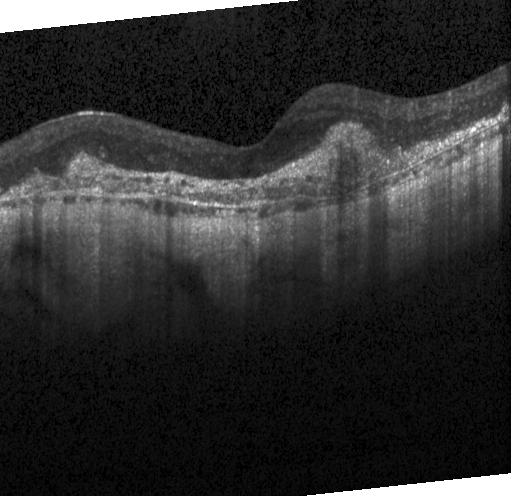 Retinal OCT B-scan, acquired on a Heidelberg Spectralis, centered on the fovea. Dx: a choroidal neovascular membrane.